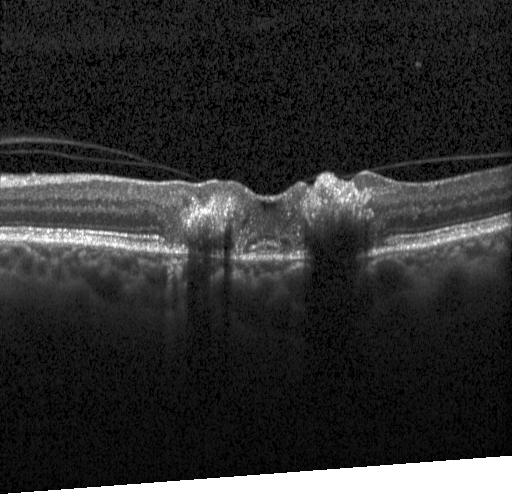

Optical coherence tomography B-scan.
Diagnosis: CNV.